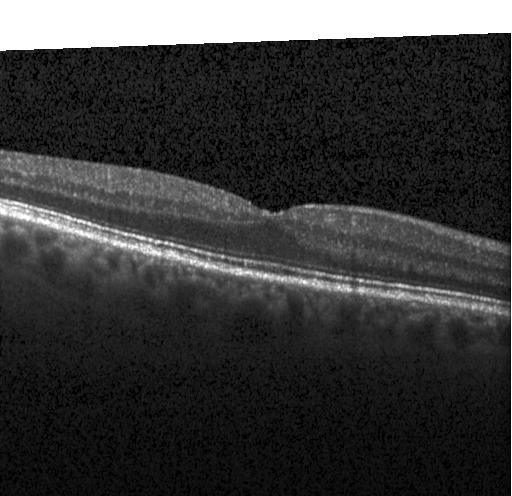
OCT finding: no CNV, no DME, and no drusen.